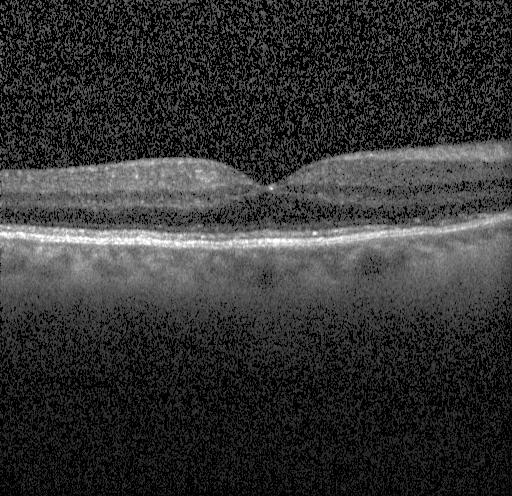 Macular OCT demonstrating neither choroidal neovascularization, diabetic macular edema, nor drusen.